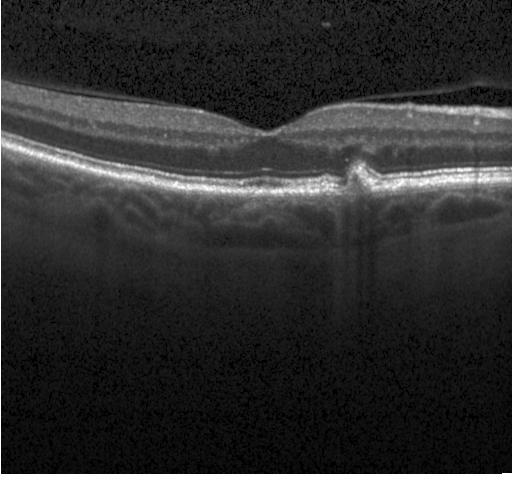 Macular OCT demonstrating multiple drusen.